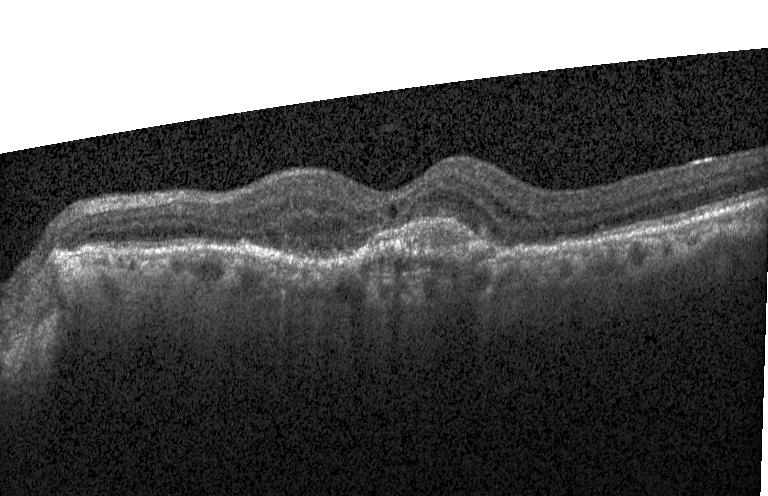
Finding: a choroidal neovascular membrane.